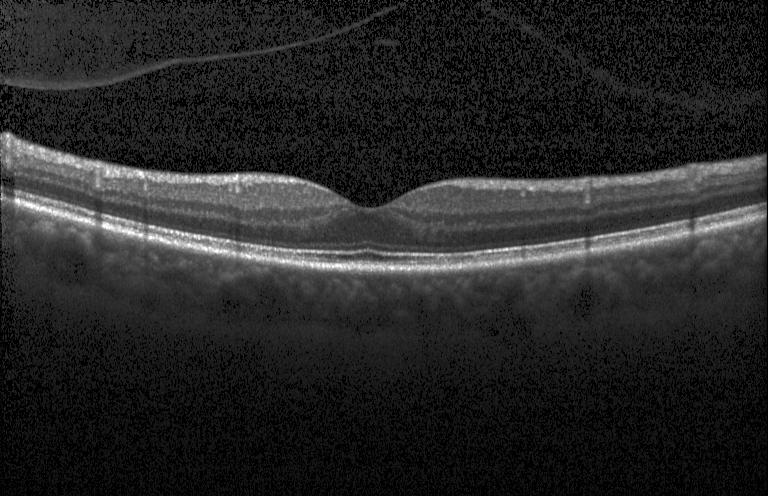
OCT B-scan — OCT finding: neither choroidal neovascularization, diabetic macular edema, nor drusen.